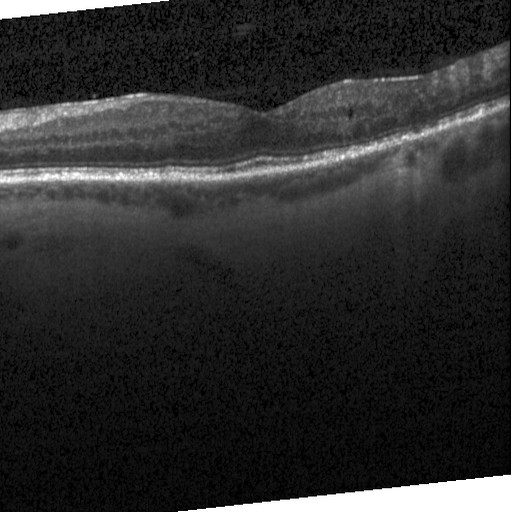

Acquired on a Heidelberg Spectralis; optical coherence tomography B-scan
Dx: diabetic macular edema.